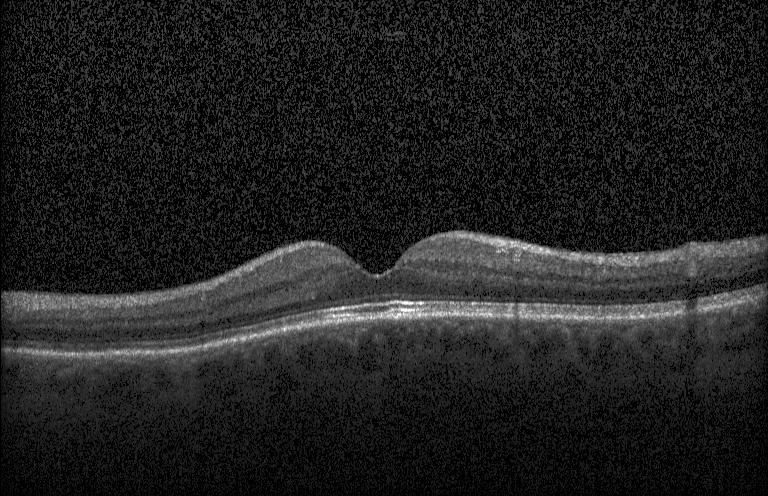 Spectral-domain OCT B-scan: no CNV, no DME, and no drusen.